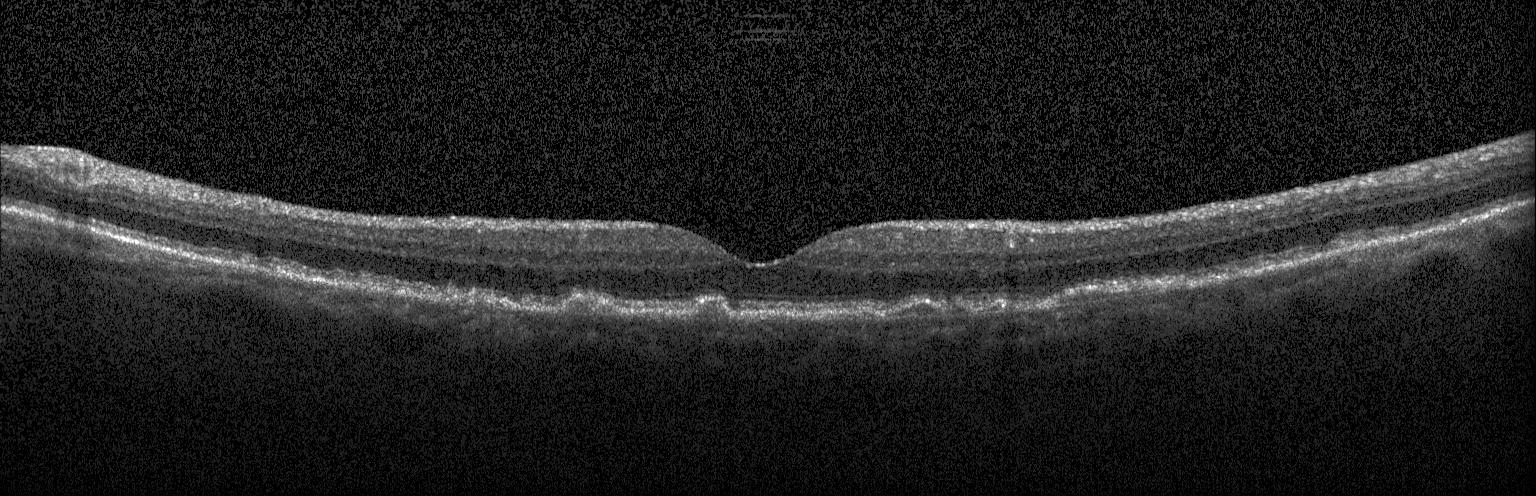 Spectral-domain OCT B-scan: multiple drusen.